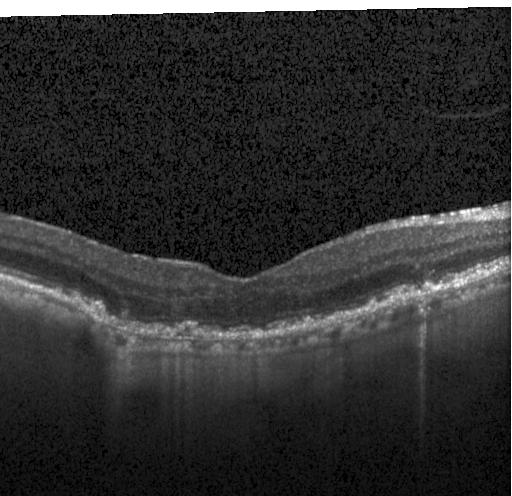 Horizontal scan through the fovea; spectral-domain OCT; optical coherence tomography scan — Macular OCT: a choroidal neovascular membrane.